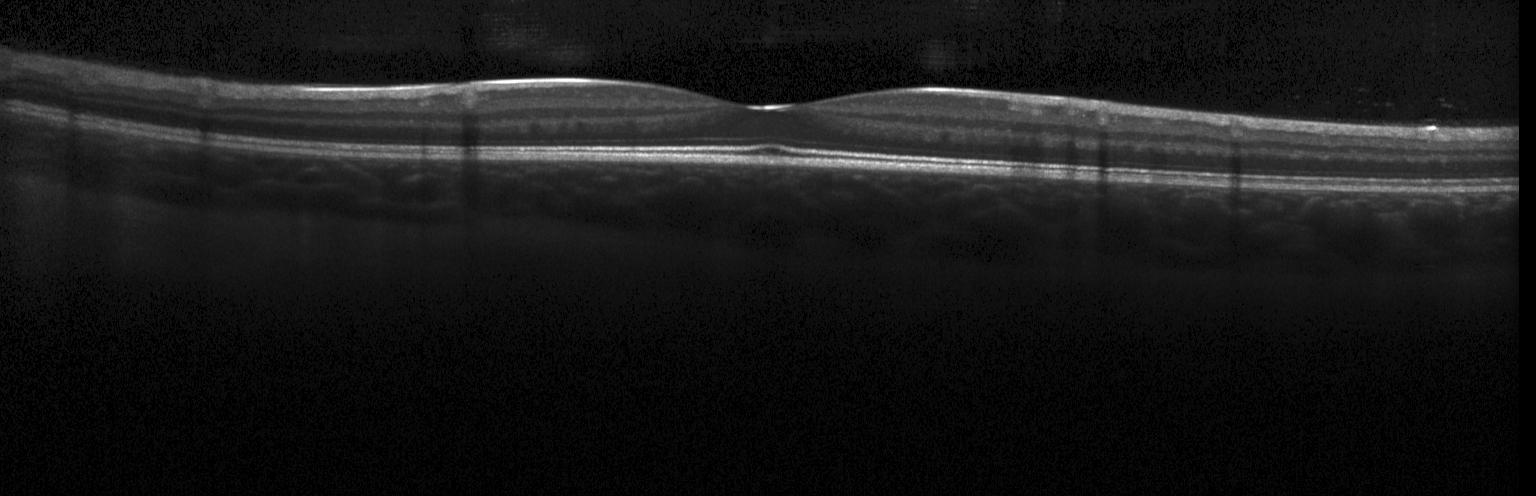

OCT scan showing no choroidal neovascularization, diabetic macular edema, or drusen.